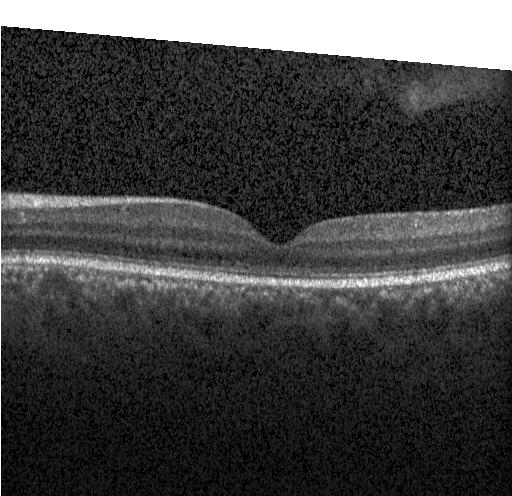

Dx: no evidence of choroidal neovascularization, diabetic macular edema, or drusen.